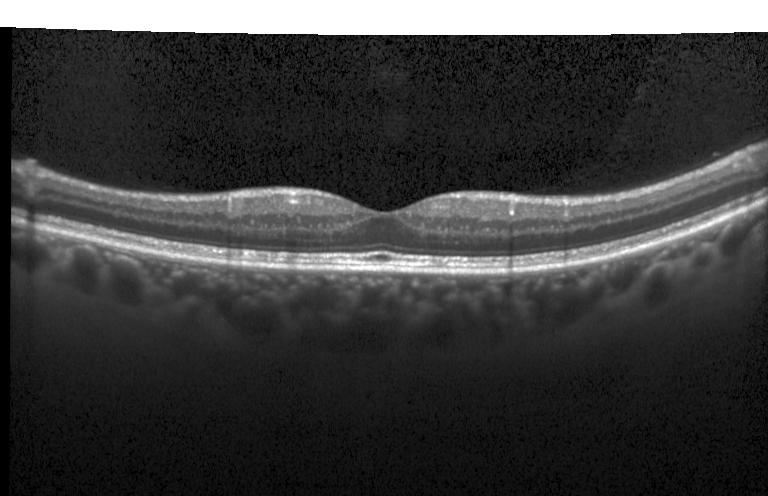

Through the macula. SD-OCT. Heidelberg Spectralis. OCT line scan — The scan shows neither CNV, DME, nor drusen.